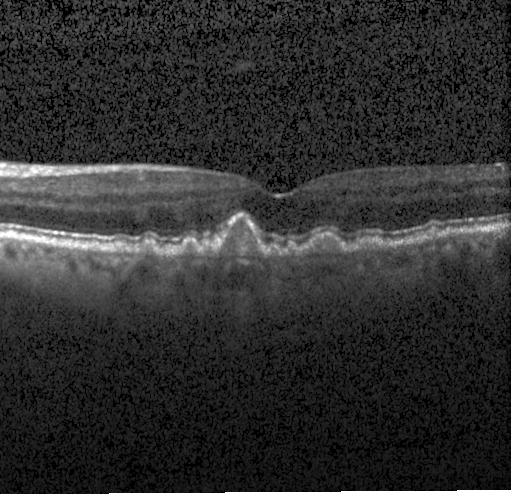

Through the macula · retinal OCT B-scan. Finding: sub-RPE drusenoid deposits.